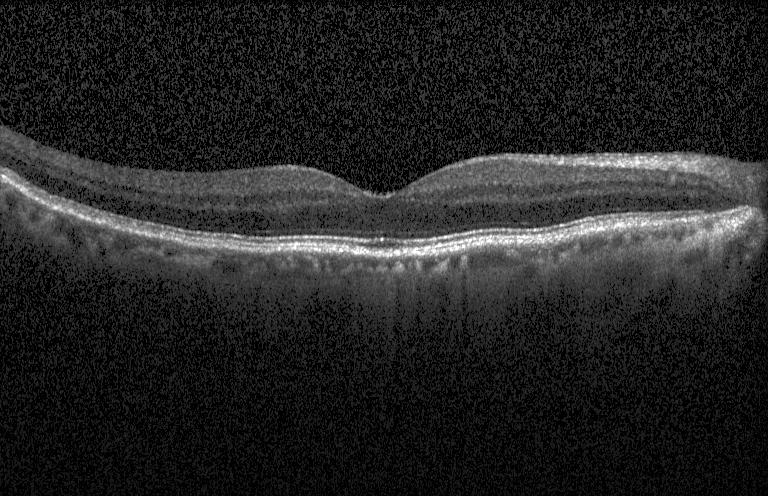

Spectral-domain OCT · OCT line scan · fovea-centered
Finding: no evidence of choroidal neovascularization, diabetic macular edema, or drusen.